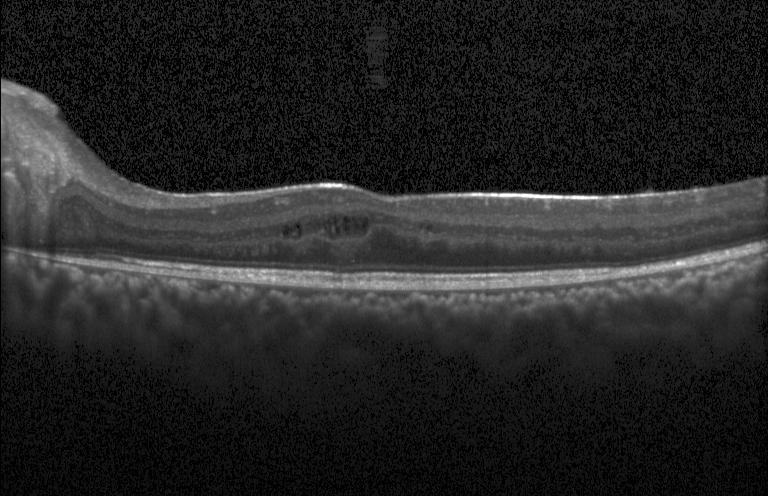 Diagnosis: diabetic macular edema.